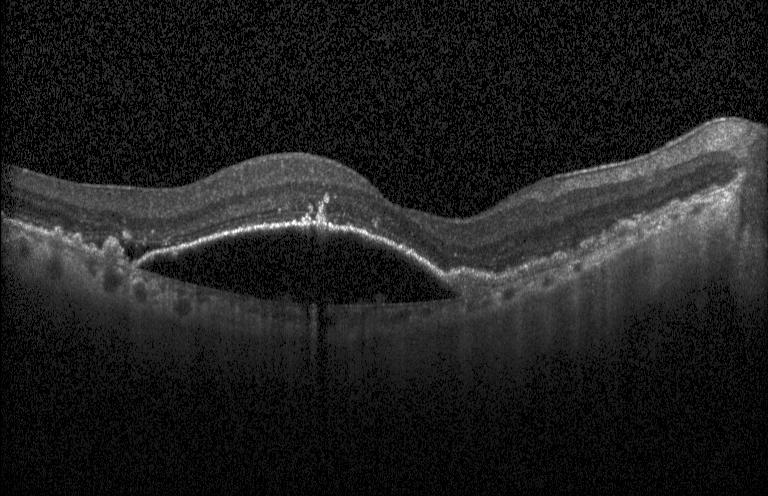

Choroidal neovascularization.